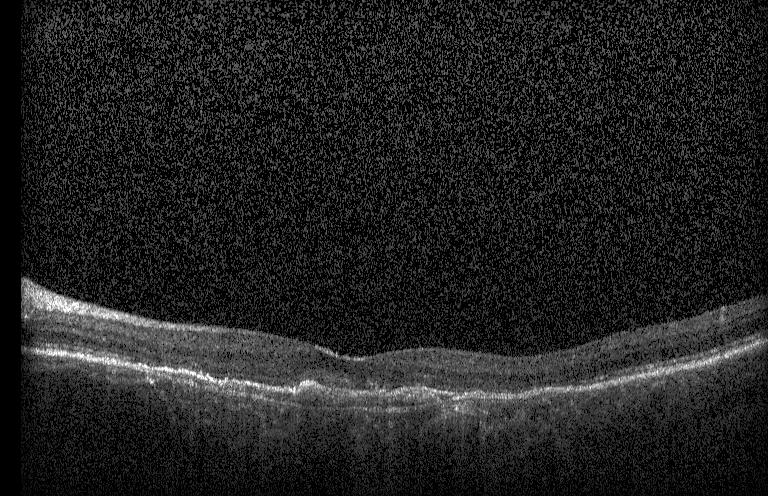
OCT B-scan; acquired on a Heidelberg Spectralis — Assessment: a choroidal neovascular membrane.